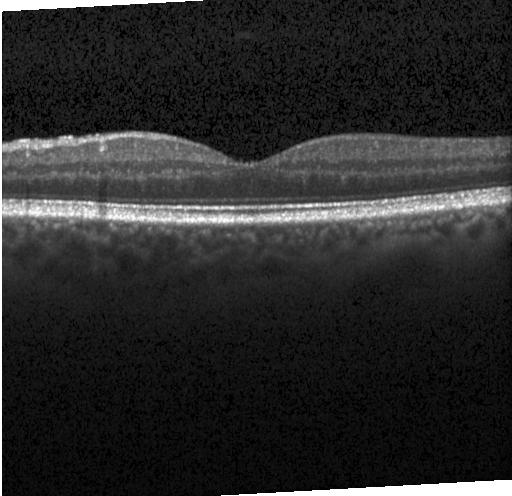
Optical coherence tomography scan. Impression: no choroidal neovascularization, diabetic macular edema, or drusen.